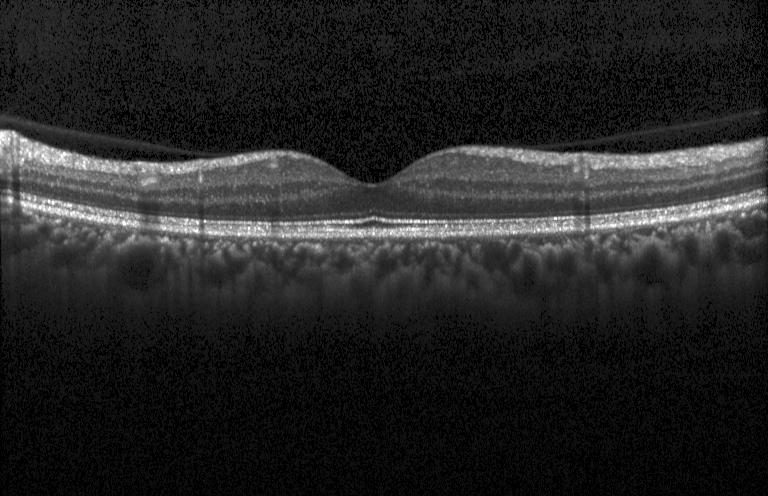

Optical coherence tomography B-scan. Centered on the fovea. SD-OCT
Diagnosis: no evidence of CNV, DME, or drusen.